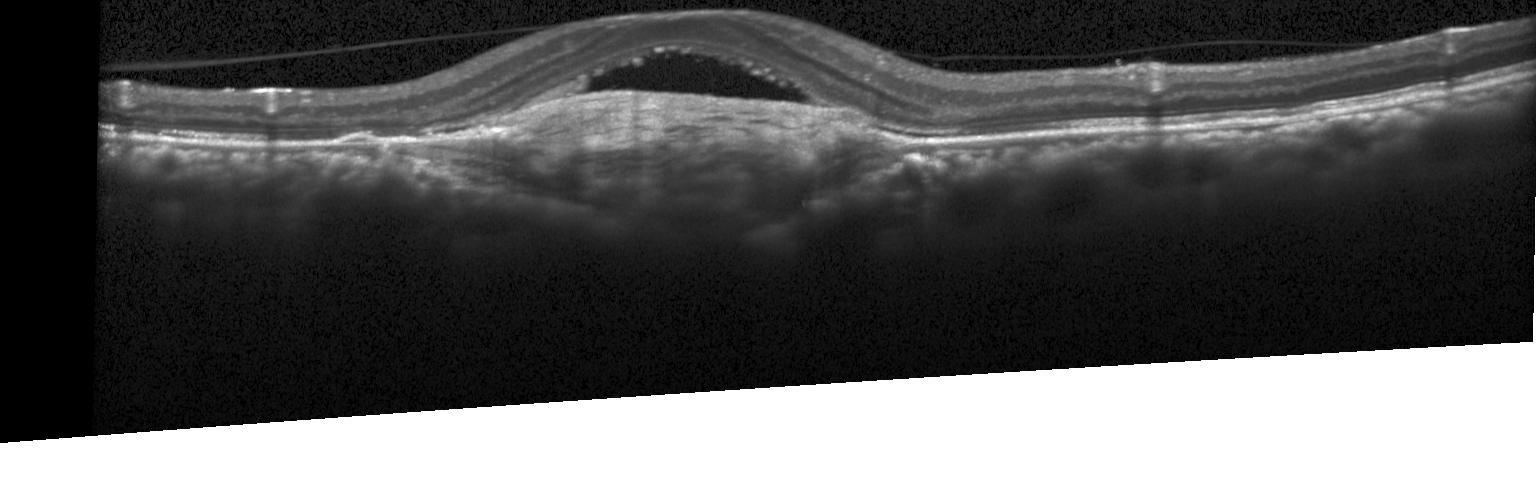 Spectral-domain optical coherence tomography · macular scan · Heidelberg Spectralis · optical coherence tomography B-scan
Finding: a choroidal neovascular membrane.